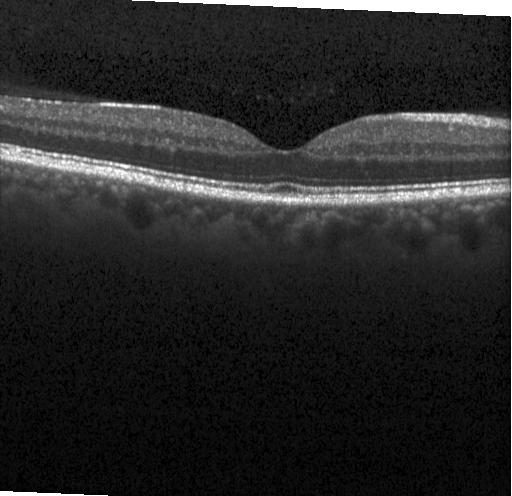
OCT line scan
Diagnosis: neither choroidal neovascularization, diabetic macular edema, nor drusen.